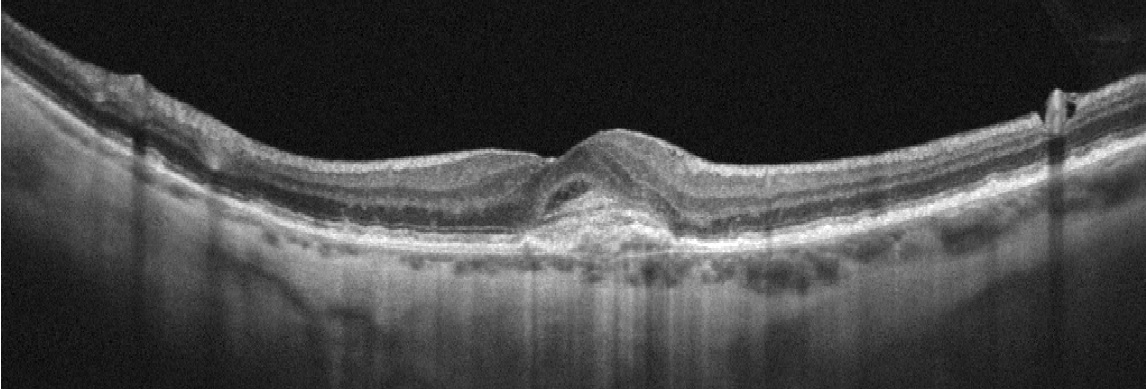 OCT line scan
Diagnosis: age-related macular degeneration (AMD).